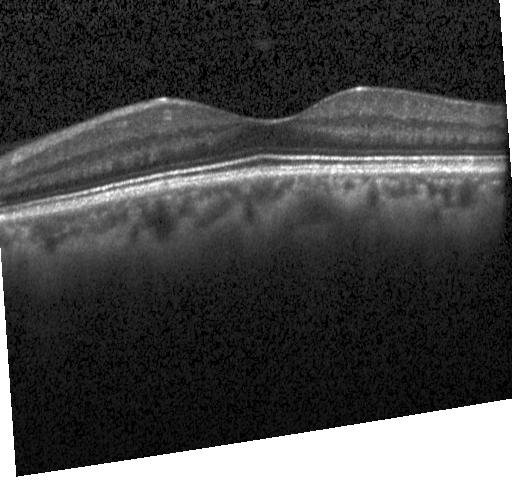 OCT B-scan — Macular OCT: no choroidal neovascularization, no diabetic macular edema, and no drusen.